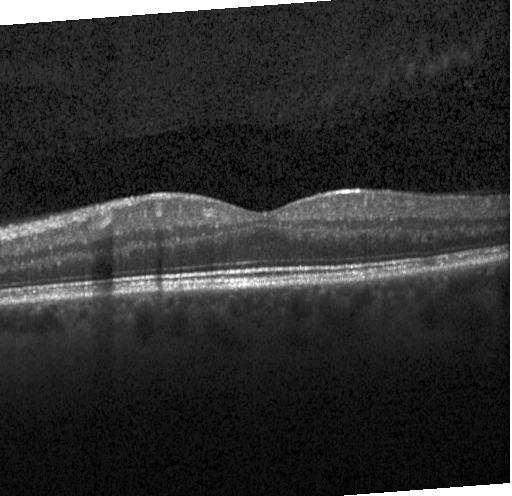 SD-OCT, optical coherence tomography scan, acquired on a Heidelberg Spectralis
Assessment: no evidence of choroidal neovascularization, diabetic macular edema, or drusen.